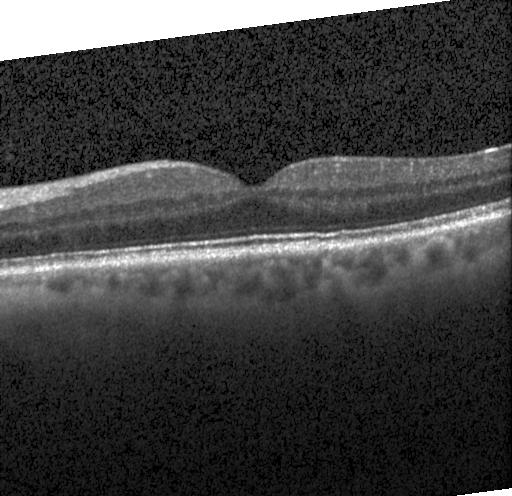

OCT line scan
This B-scan demonstrates no evidence of CNV, DME, or drusen.